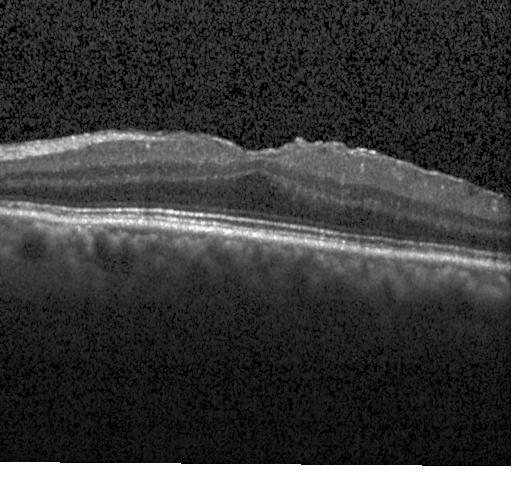 Optical coherence tomography scan, SD-OCT
Finding: no choroidal neovascularization, no diabetic macular edema, and no drusen.